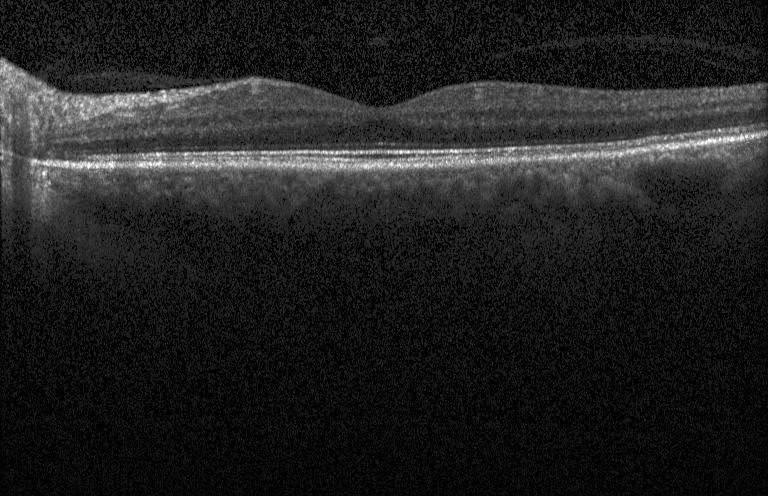

OCT line scan.
This B-scan demonstrates no choroidal neovascularization, diabetic macular edema, or drusen.